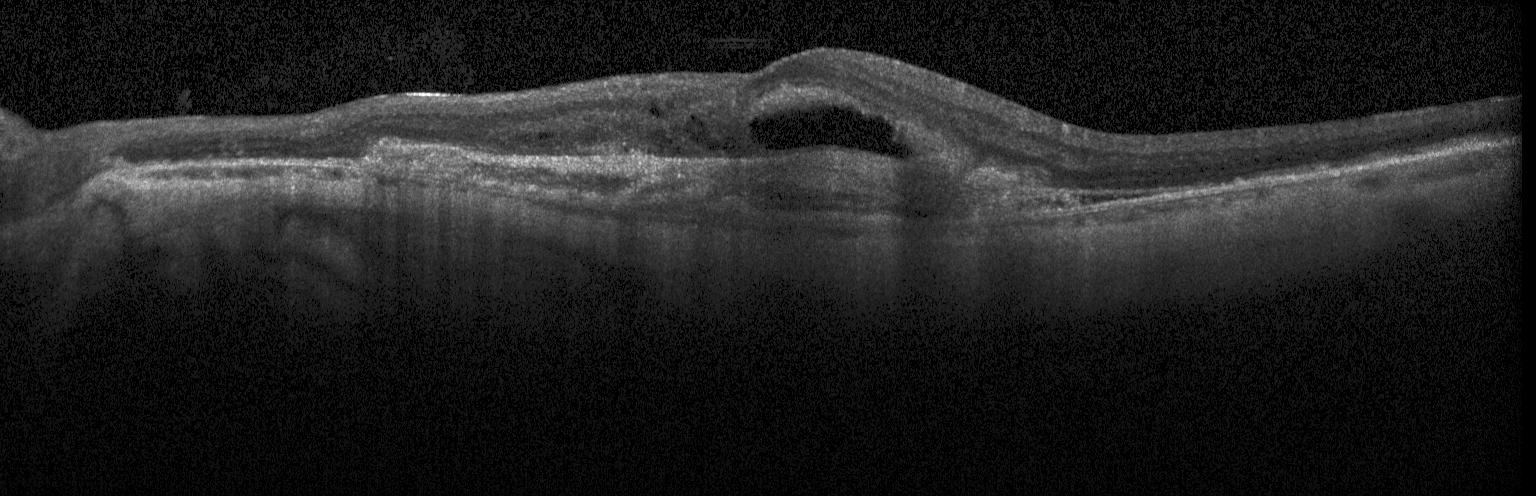
Retinal OCT B-scan; through the macula — Dx: a choroidal neovascular membrane.